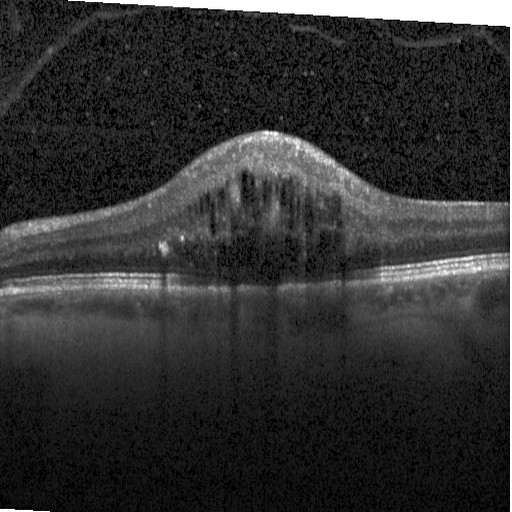 The scan shows DME.